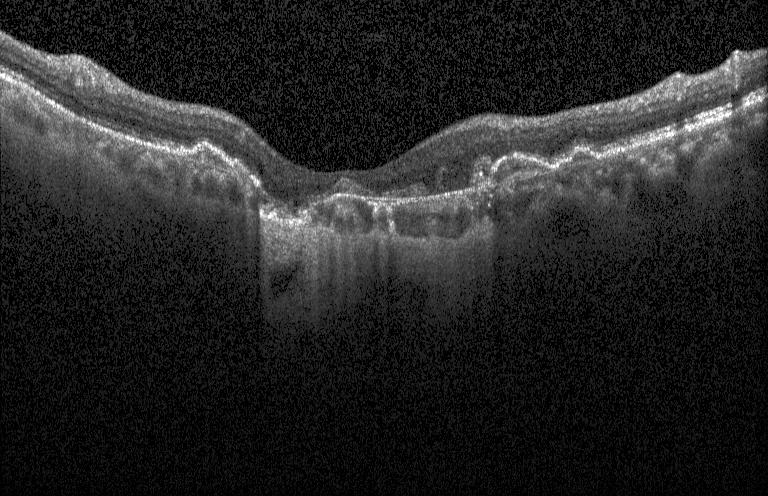 Retinal OCT B-scan. A choroidal neovascular membrane.